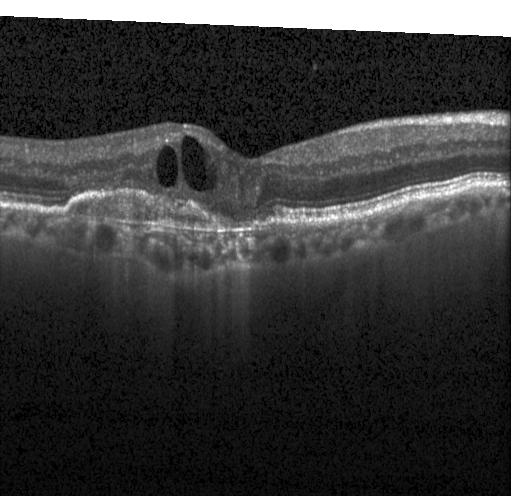
Spectral-domain OCT B-scan: CNV.